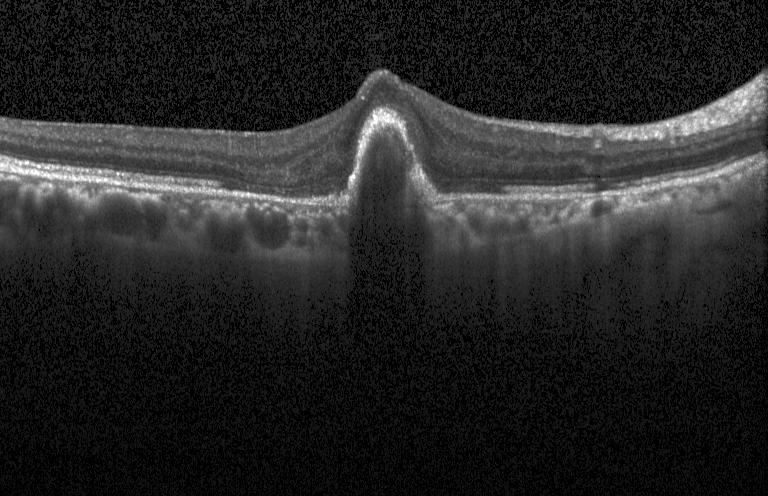 Finding: a choroidal neovascular membrane.